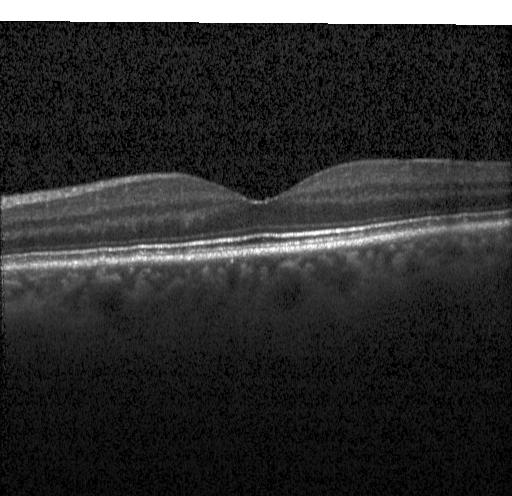
Impression: no evidence of choroidal neovascularization, diabetic macular edema, or drusen.